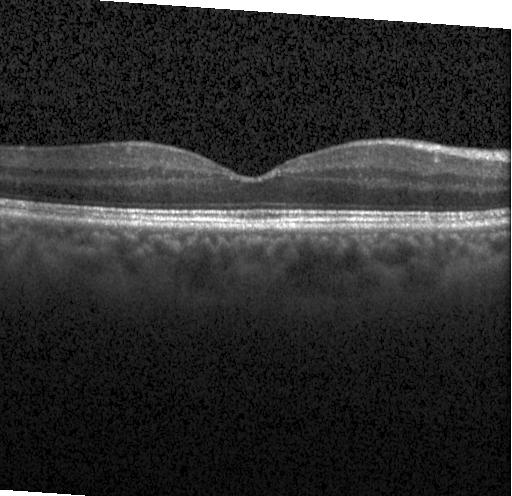 Spectral-domain OCT. Acquired on a Heidelberg Spectralis. Horizontal scan through the fovea. OCT B-scan — This B-scan demonstrates neither choroidal neovascularization, diabetic macular edema, nor drusen.